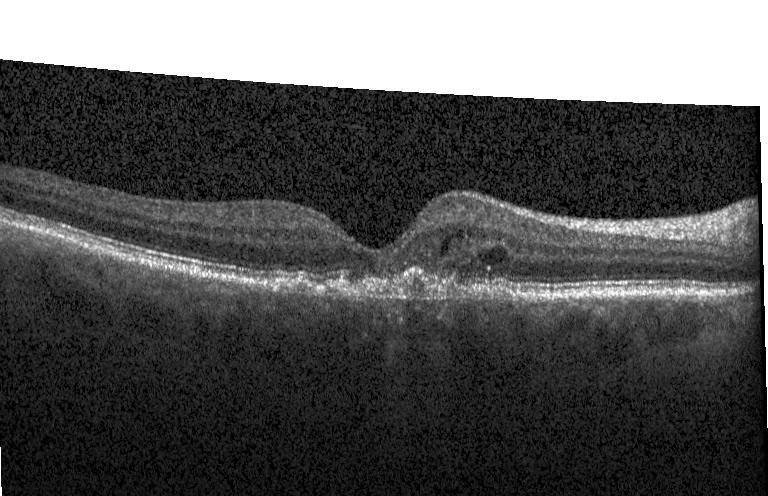

Impression: a choroidal neovascular membrane.